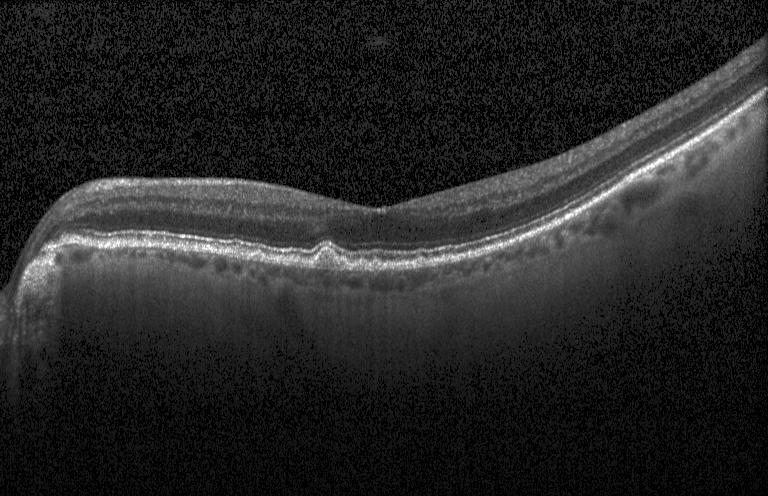 Optical coherence tomography scan · fovea-centered
Dx: multiple drusen.